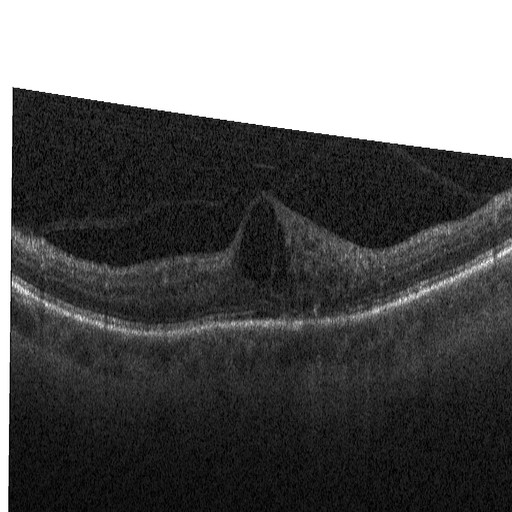
The scan shows diabetic macular edema.